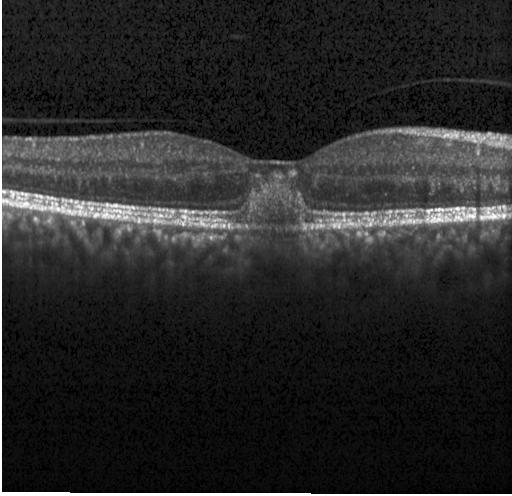 Retinal OCT cross-section showing choroidal neovascularization.